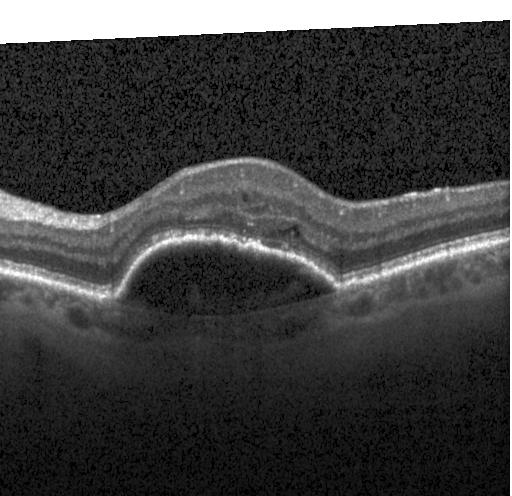

Macular scan. Heidelberg Spectralis. Retinal OCT B-scan — This B-scan demonstrates choroidal neovascularization (CNV).